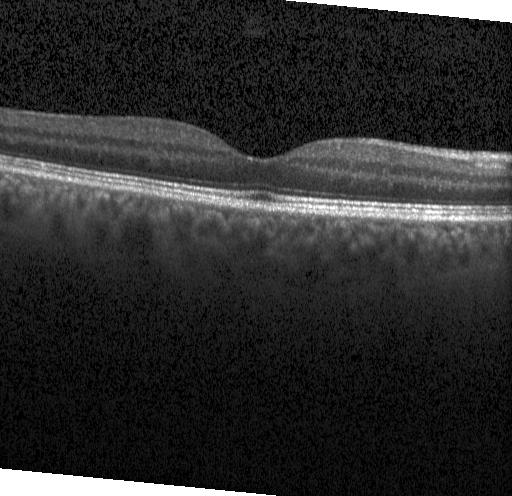

Macular OCT demonstrating no evidence of choroidal neovascularization, diabetic macular edema, or drusen.